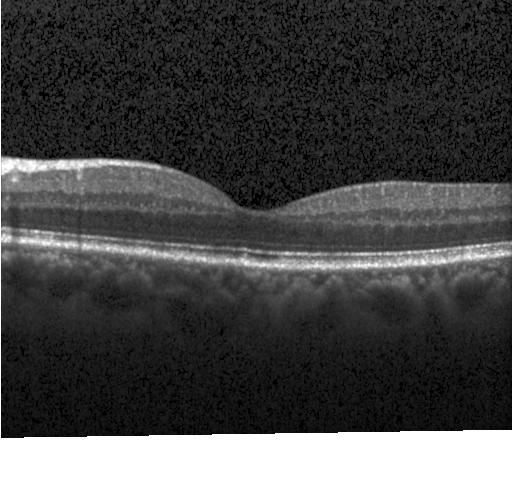

OCT scan showing no choroidal neovascularization, diabetic macular edema, or drusen.